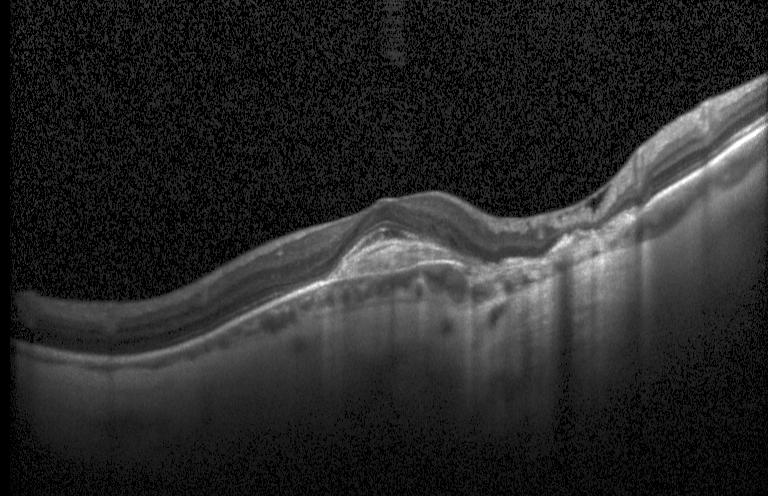 Spectral-domain optical coherence tomography, Heidelberg Spectralis OCT system, optical coherence tomography B-scan — Impression: choroidal neovascularization.